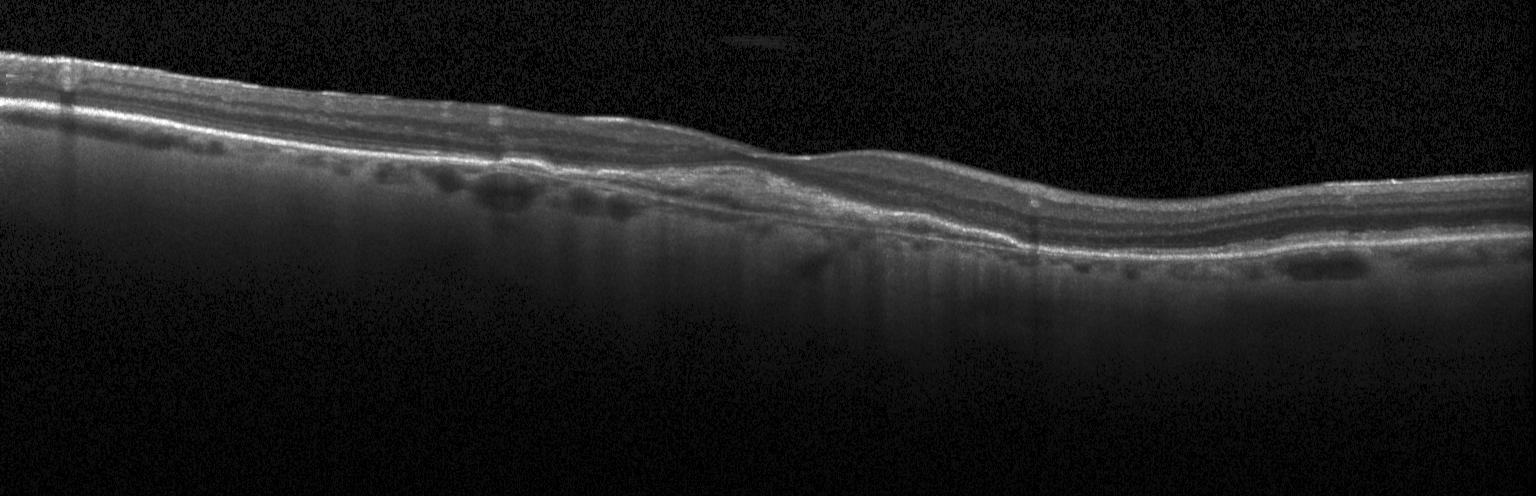 OCT B-scan. Macular scan — Finding: CNV.